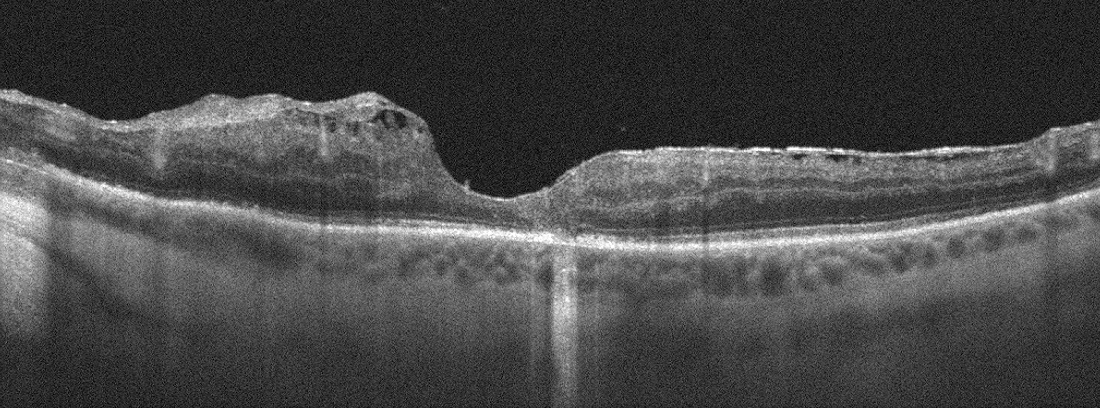 Diagnosis: DME.